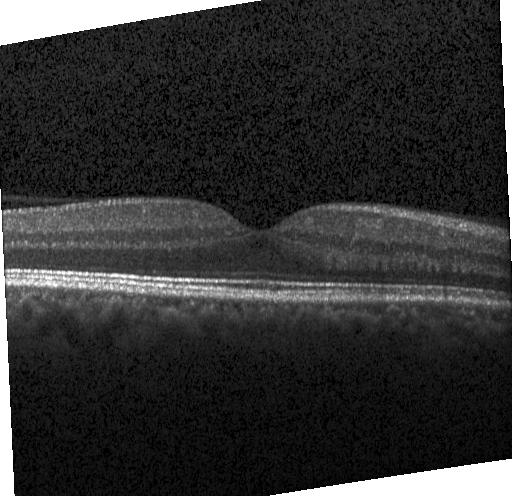
OCT scan showing no evidence of CNV, DME, or drusen.